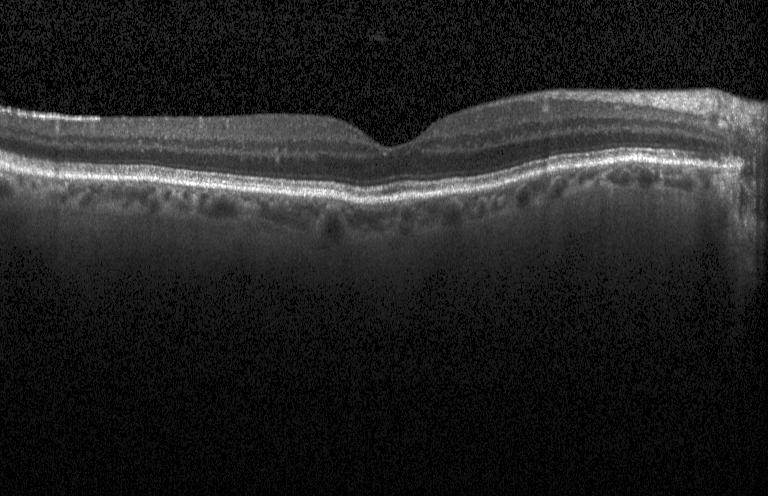 Assessment: no evidence of CNV, DME, or drusen.